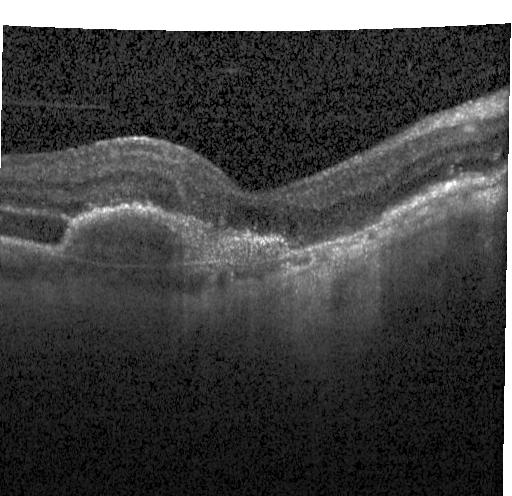
Retinal OCT B-scan · acquired on a Heidelberg Spectralis · fovea-centered.
OCT finding: choroidal neovascularization (CNV).